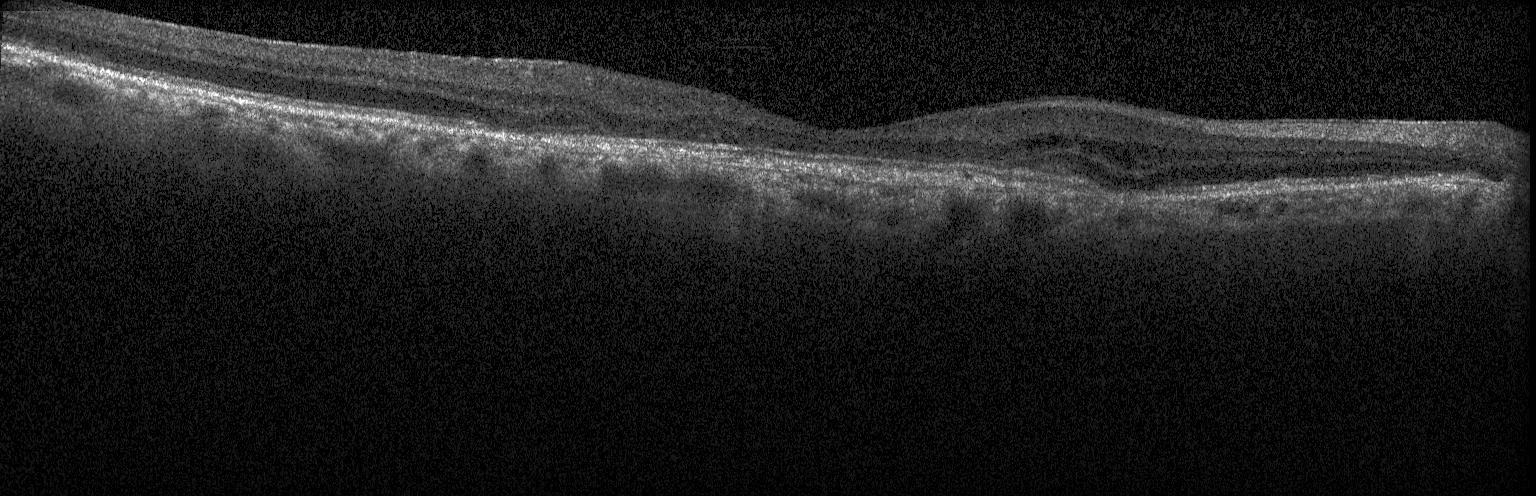
Spectral-domain OCT · OCT line scan · centered on the fovea.
Dx: a choroidal neovascular membrane.